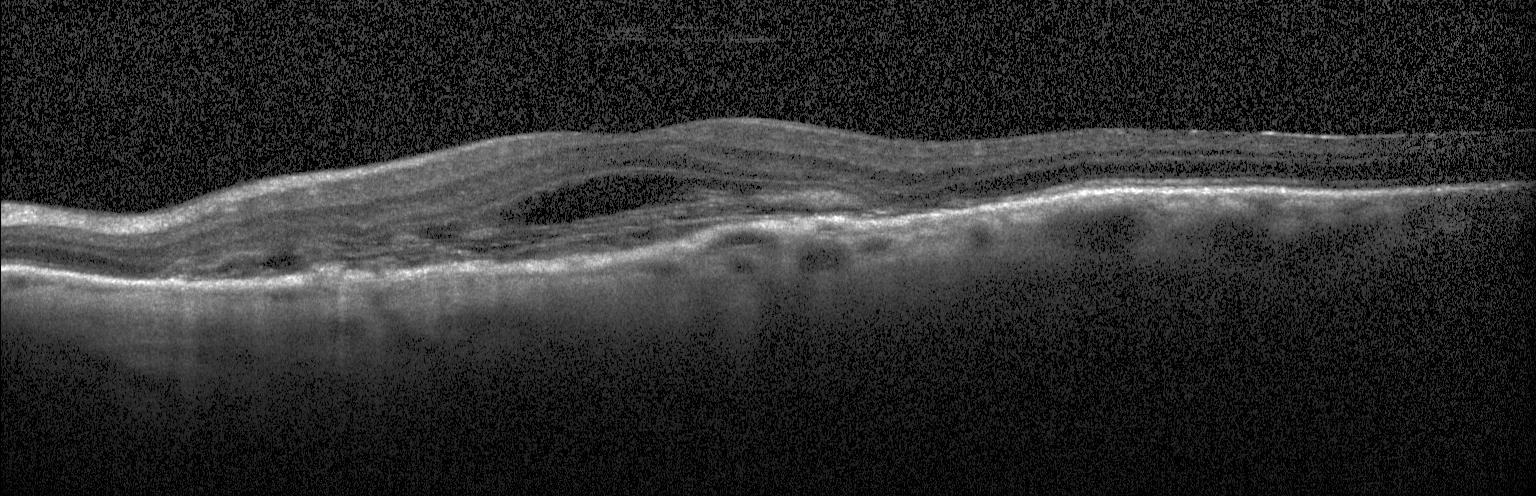 OCT B-scan — Finding: a choroidal neovascular membrane.